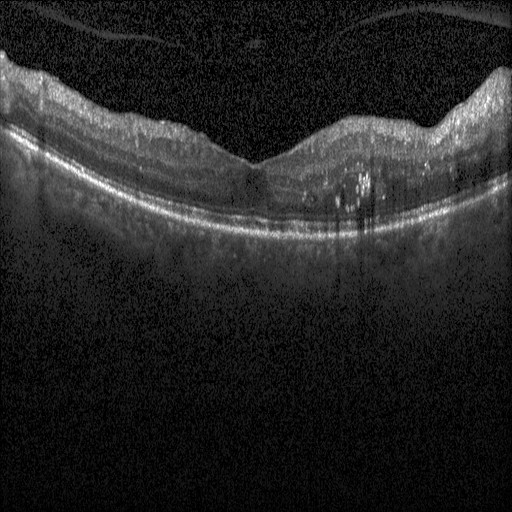 Optical coherence tomography scan. Spectral-domain optical coherence tomography — Finding: diabetic macular edema (DME).